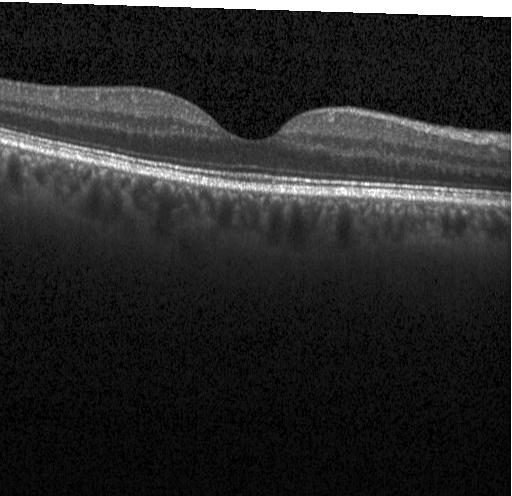

Horizontal scan through the fovea, spectral-domain OCT, OCT line scan. The scan shows neither choroidal neovascularization, diabetic macular edema, nor drusen.